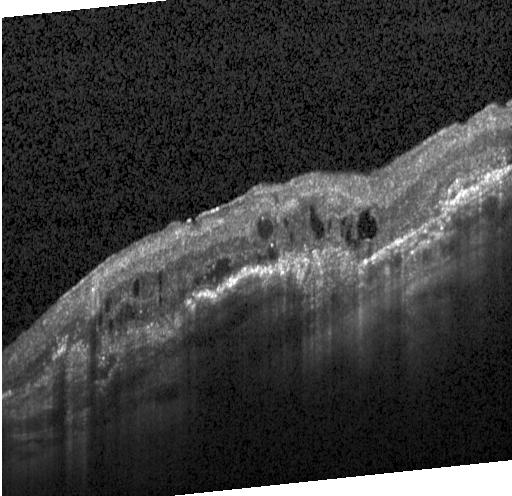
Impression: choroidal neovascularization.